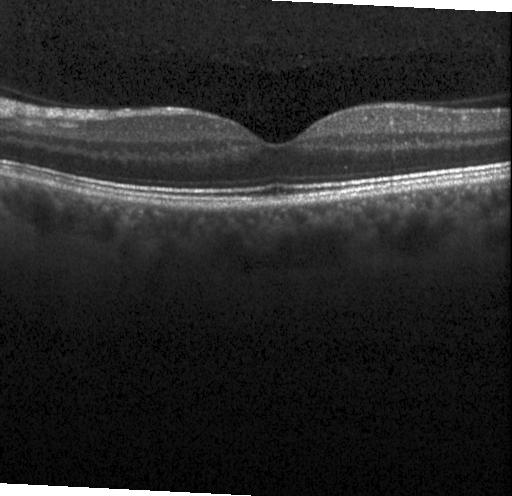
Spectral-domain OCT. Optical coherence tomography scan. Heidelberg Spectralis OCT system. Through the macula.
Diagnosis: no choroidal neovascularization, no diabetic macular edema, and no drusen.